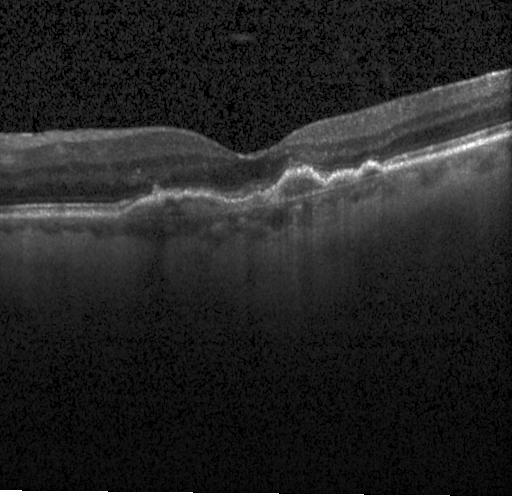

Spectral-domain OCT B-scan: a choroidal neovascular membrane.